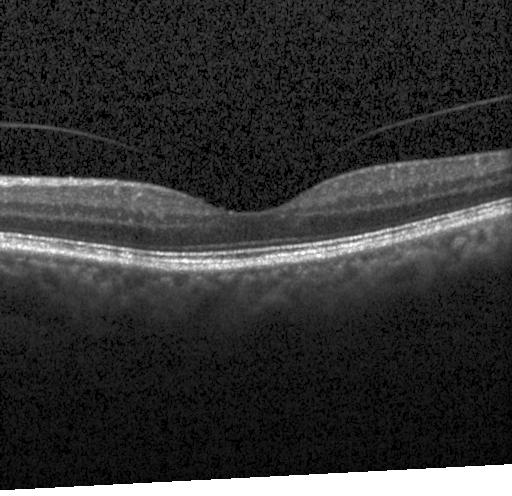 Acquired on a Heidelberg Spectralis · OCT B-scan
Diagnosis: neither CNV, DME, nor drusen.